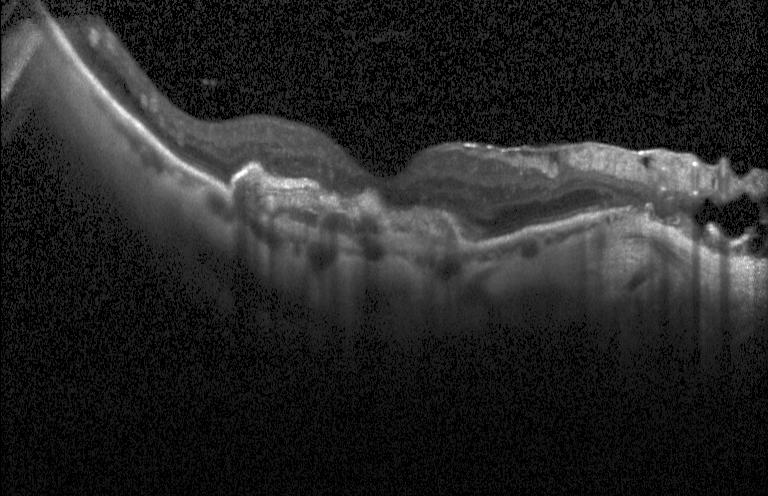
Impression: a choroidal neovascular membrane.